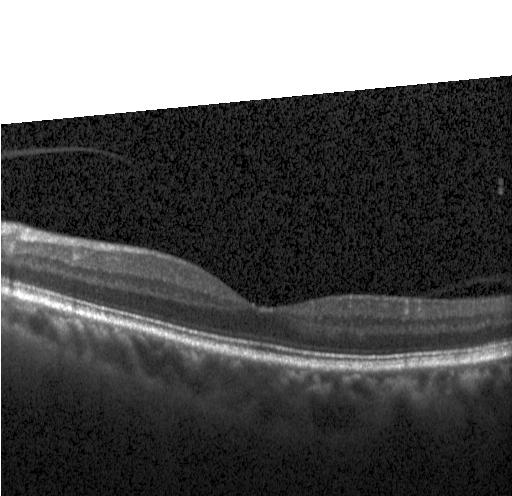

Retinal OCT cross-section. Heidelberg Spectralis. Fovea-centered. Spectral-domain optical coherence tomography
OCT finding: neither choroidal neovascularization, diabetic macular edema, nor drusen.